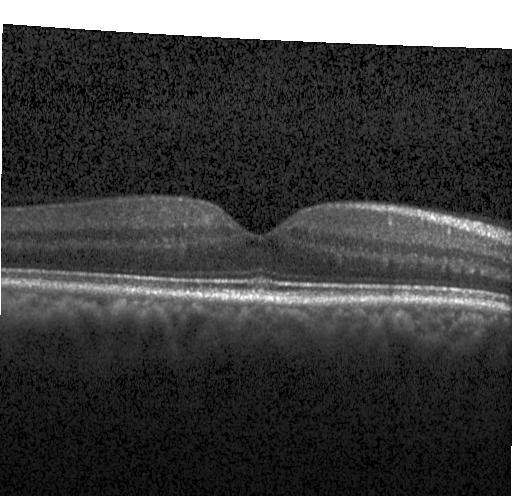

OCT line scan · spectral-domain OCT · through the macula. No CNV, DME, or drusen.